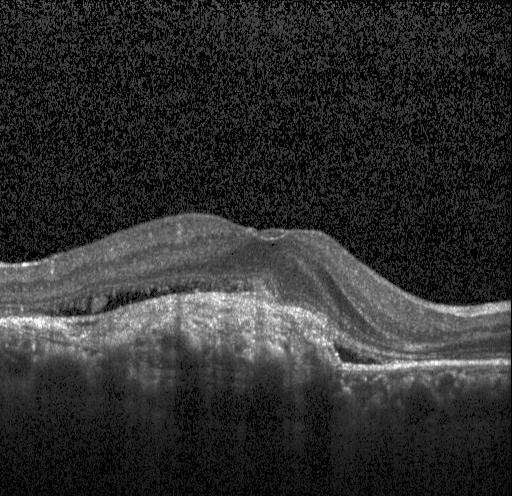 Optical coherence tomography B-scan; instrument: Heidelberg Spectralis. Impression: a choroidal neovascular membrane.